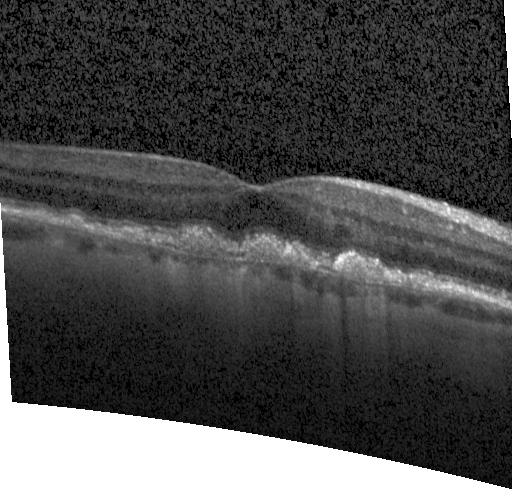 Optical coherence tomography B-scan
OCT finding: CNV.